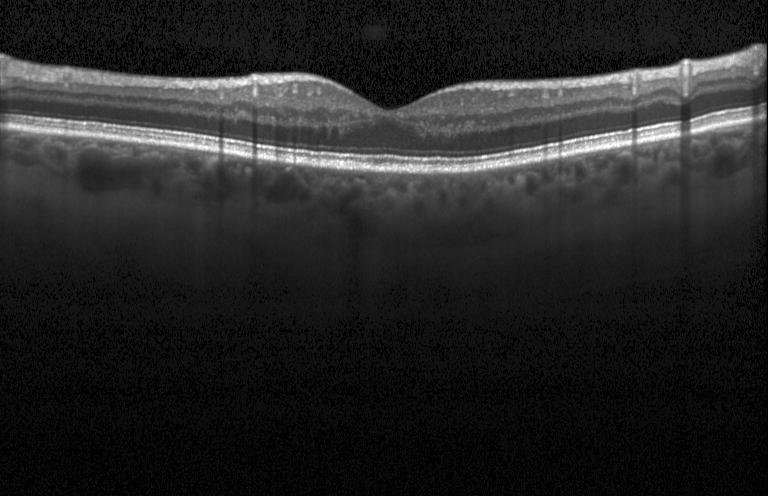

Macular OCT: no choroidal neovascularization, no diabetic macular edema, and no drusen.